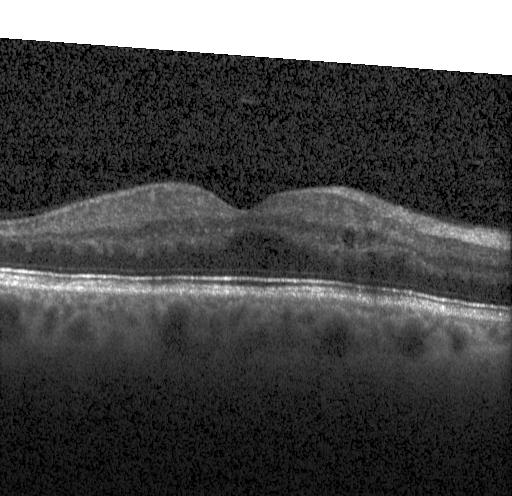 OCT finding: diabetic macular edema.